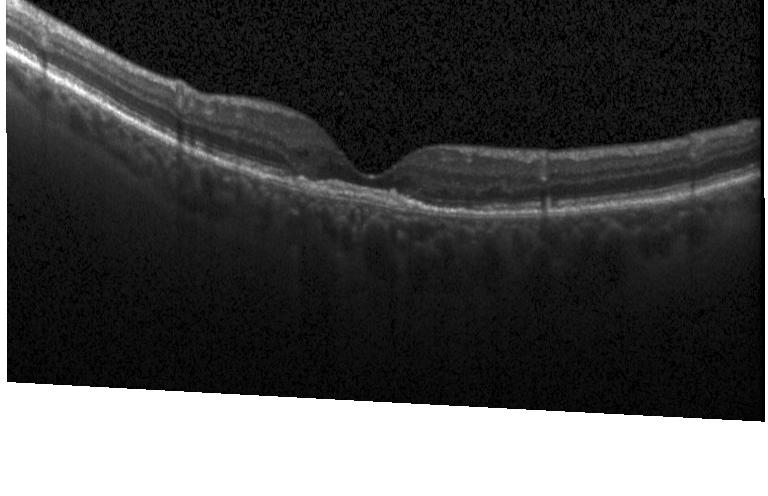 Centered on the fovea; optical coherence tomography B-scan; SD-OCT; Heidelberg Spectralis OCT system.
This B-scan demonstrates a choroidal neovascular membrane.